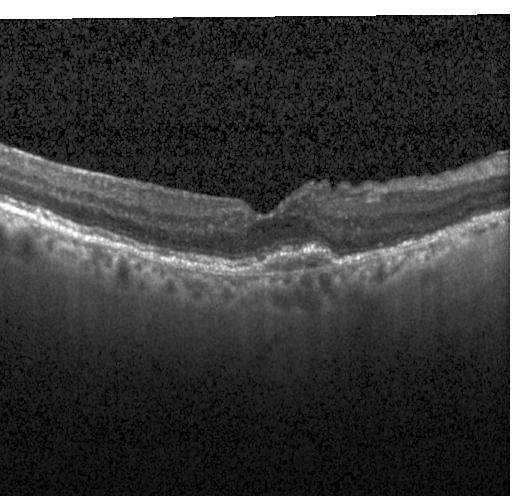
Horizontal scan through the fovea. Spectral-domain OCT. Optical coherence tomography scan — Macular OCT: a choroidal neovascular membrane.